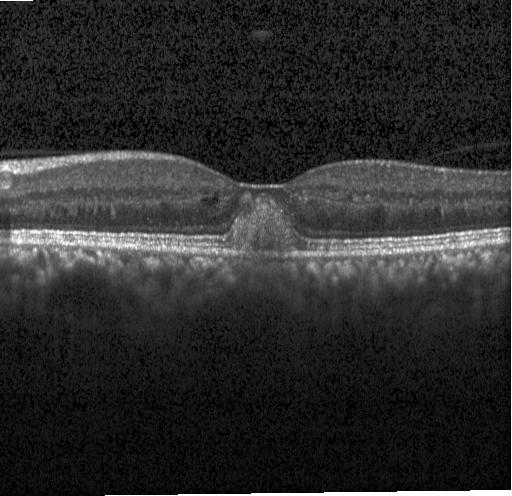

Spectral-domain OCT B-scan: a choroidal neovascular membrane.